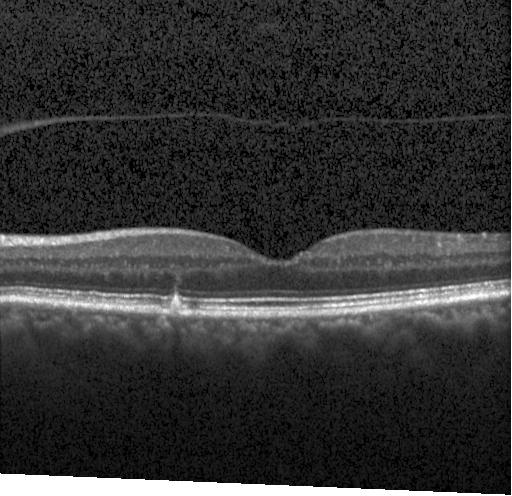

Optical coherence tomography scan — Diagnosis: multiple drusen.